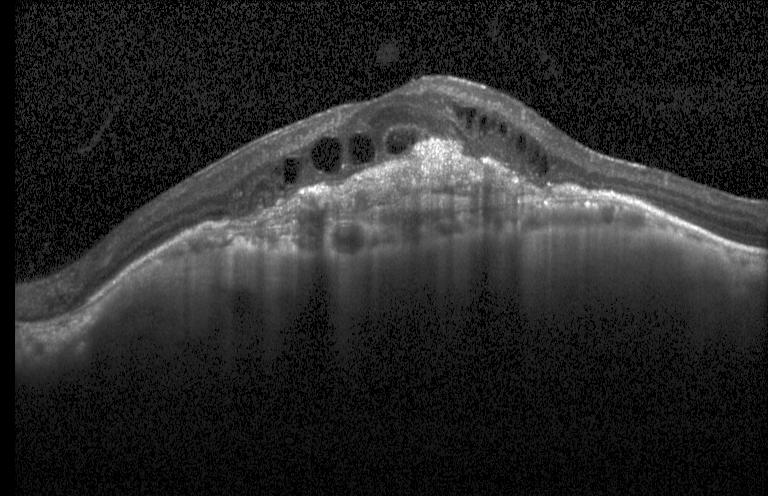 Macular OCT: a choroidal neovascular membrane.